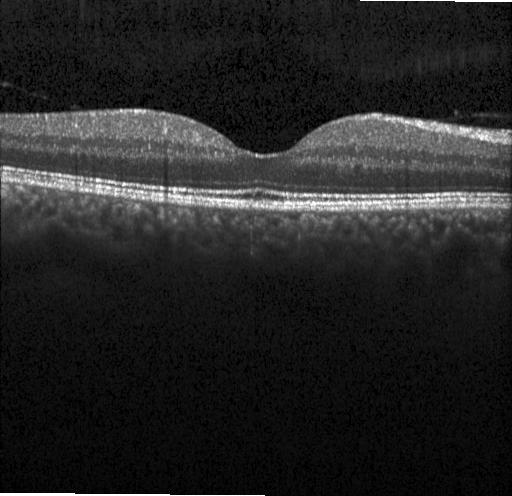 Optical coherence tomography B-scan — Assessment: no choroidal neovascularization, no diabetic macular edema, and no drusen.